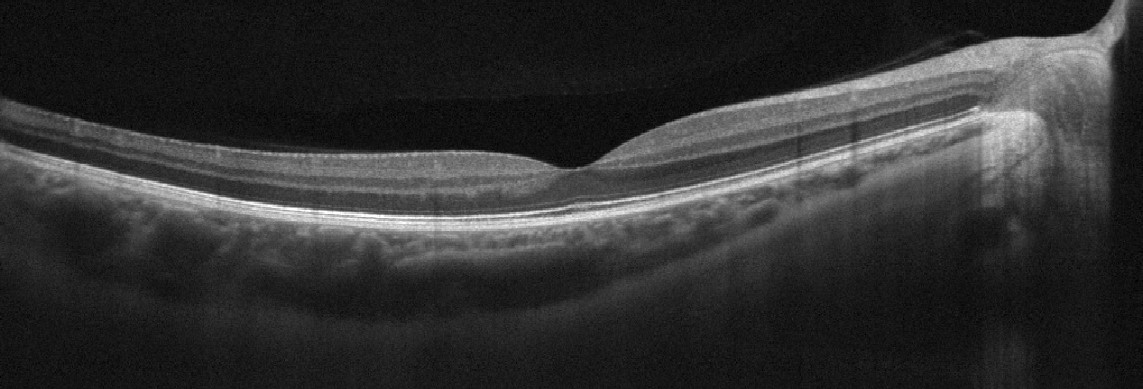
Macular OCT demonstrating no AMD, DME, ERM, RAO, RVO, or VID.